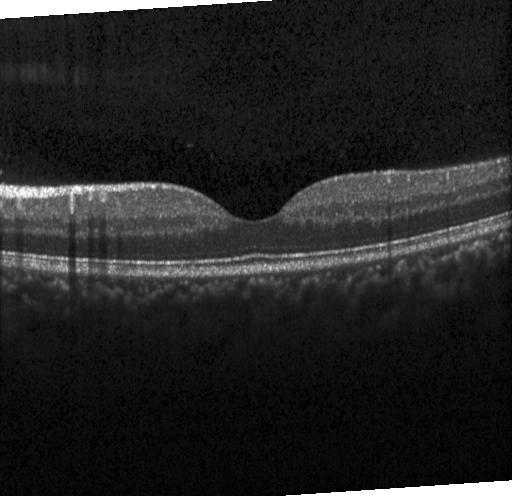

OCT finding: no evidence of choroidal neovascularization, diabetic macular edema, or drusen.